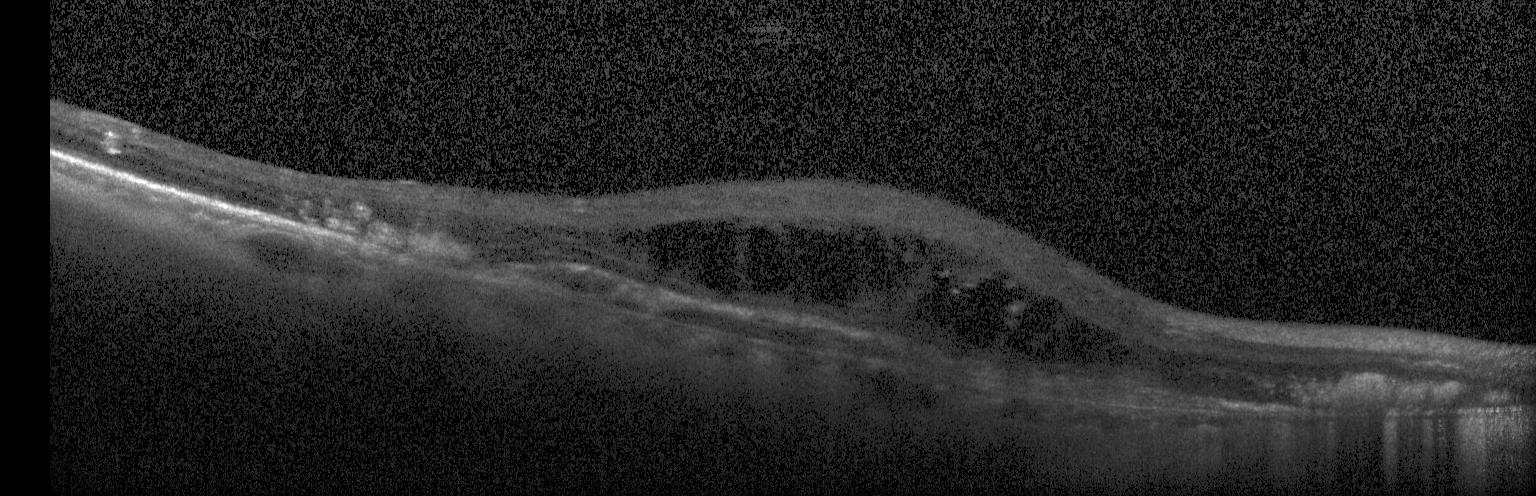

Through the macula; spectral-domain OCT; instrument: Heidelberg Spectralis; OCT line scan.
Impression: a choroidal neovascular membrane.